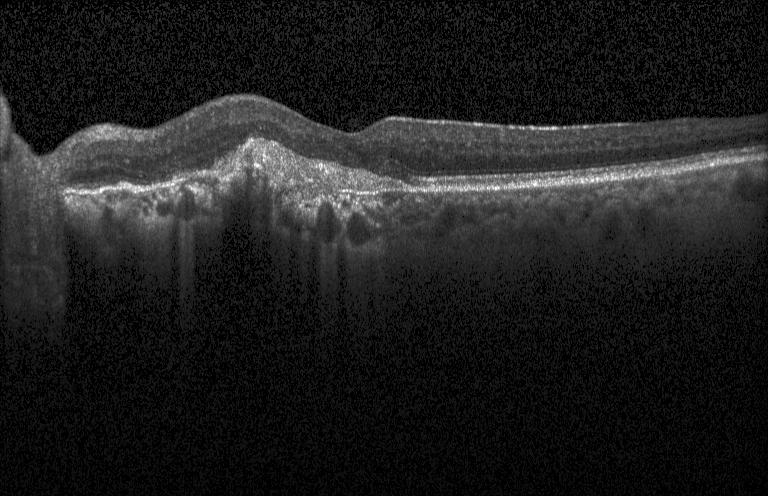
Retinal OCT cross-section. Dx: choroidal neovascularization.